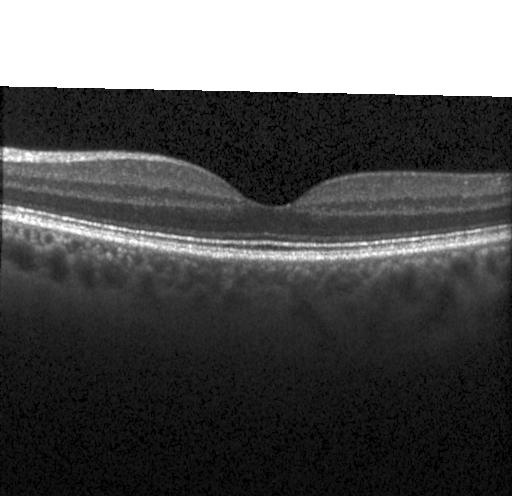
Assessment: no choroidal neovascularization, diabetic macular edema, or drusen.